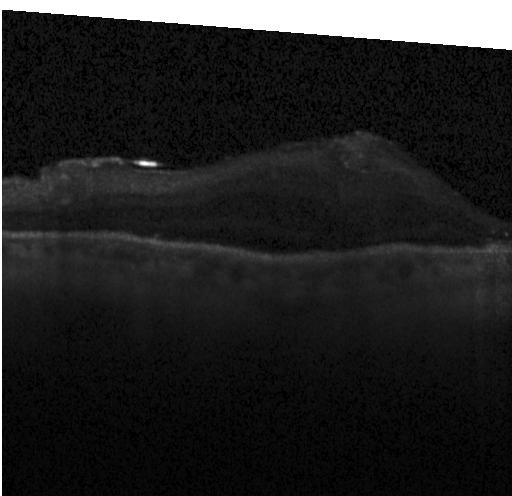

OCT B-scan showing choroidal neovascularization.